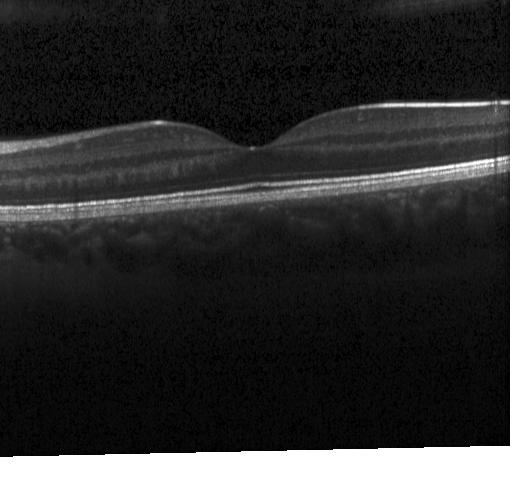
Finding: no CNV, DME, or drusen.